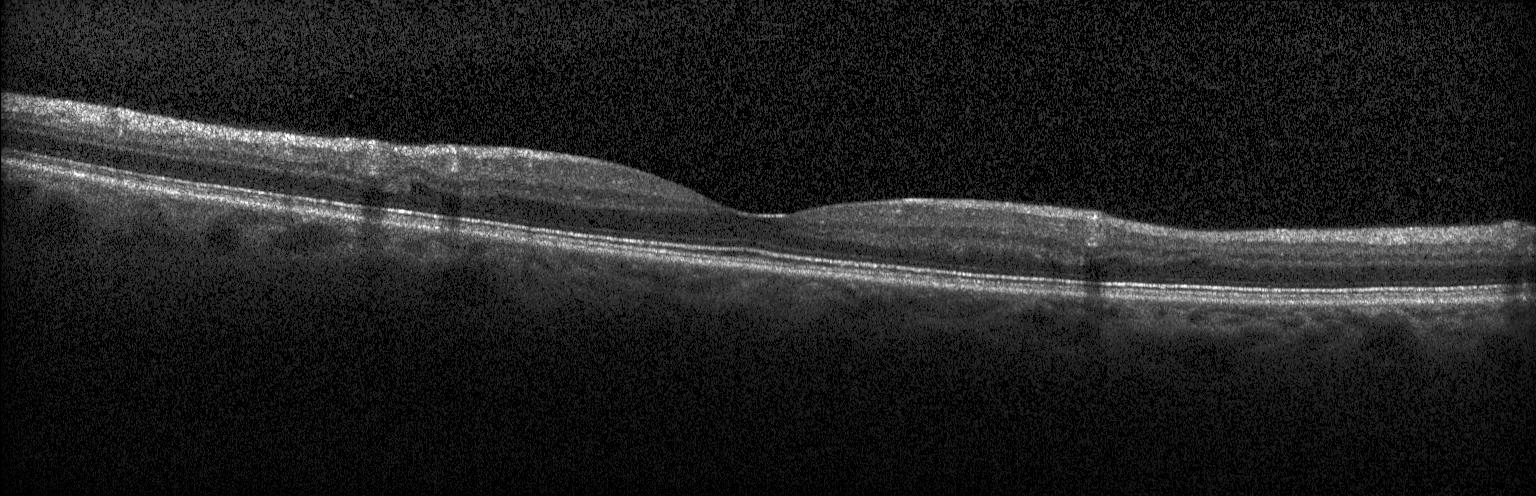

Finding: no choroidal neovascularization, diabetic macular edema, or drusen.